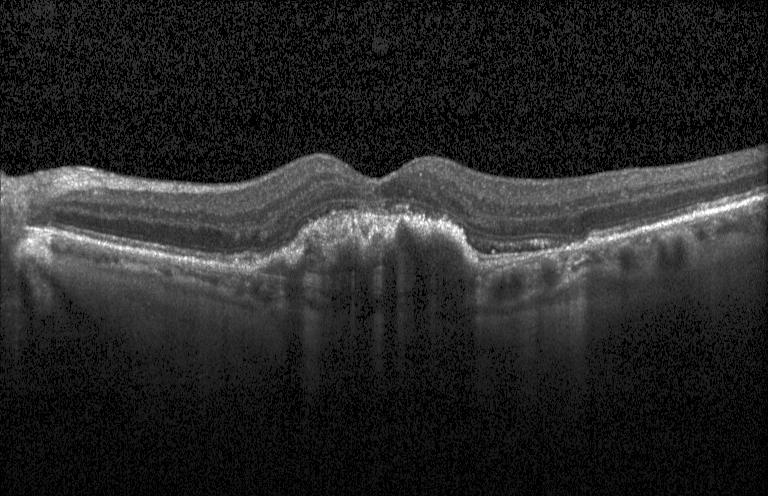

OCT finding: a choroidal neovascular membrane.